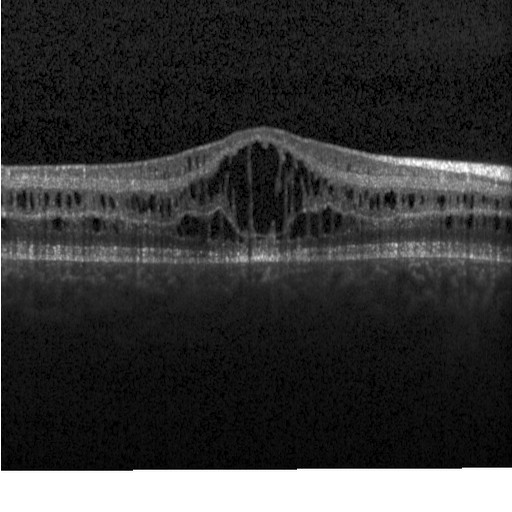
Fovea-centered · OCT line scan
Impression: diabetic macular edema (DME).